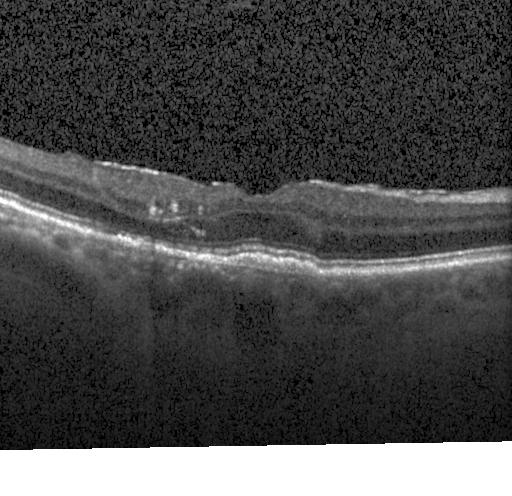 Instrument: Heidelberg Spectralis. OCT B-scan. Centered on the fovea.
This B-scan demonstrates choroidal neovascularization (CNV).